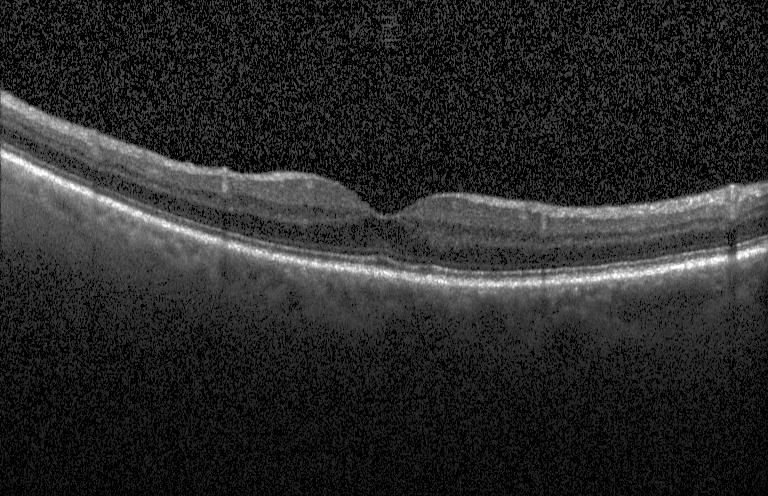 OCT line scan. Heidelberg Spectralis OCT system. SD-OCT
Finding: no evidence of CNV, DME, or drusen.